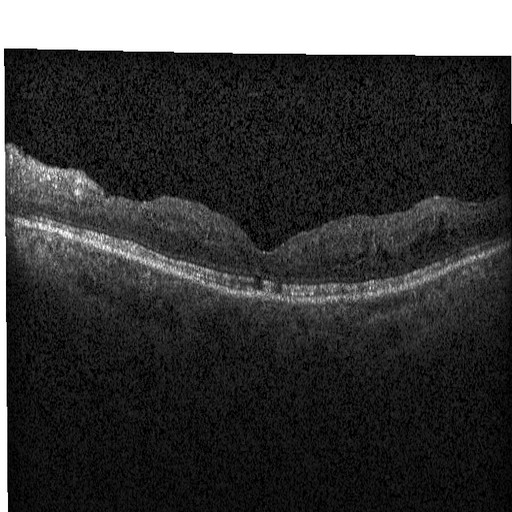 Retinal OCT B-scan · spectral-domain OCT · centered on the fovea · acquired on a Heidelberg Spectralis — This B-scan demonstrates diabetic macular edema (DME).